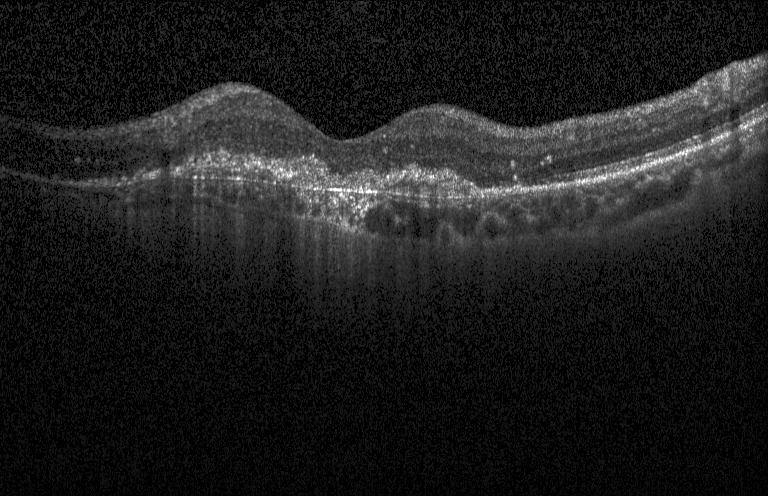

OCT line scan — Diagnosis: choroidal neovascularization.